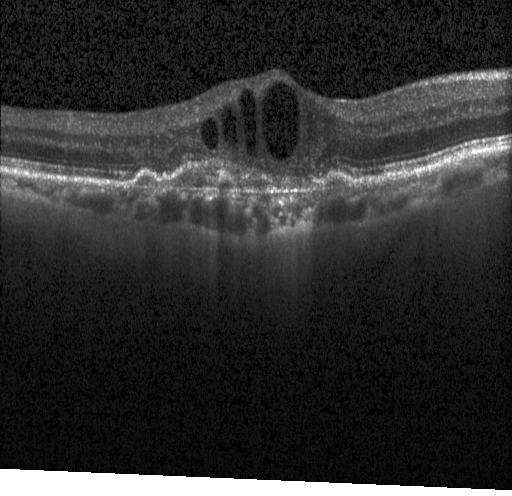

Instrument: Heidelberg Spectralis. Fovea-centered. Retinal OCT cross-section. SD-OCT — Assessment: a choroidal neovascular membrane.